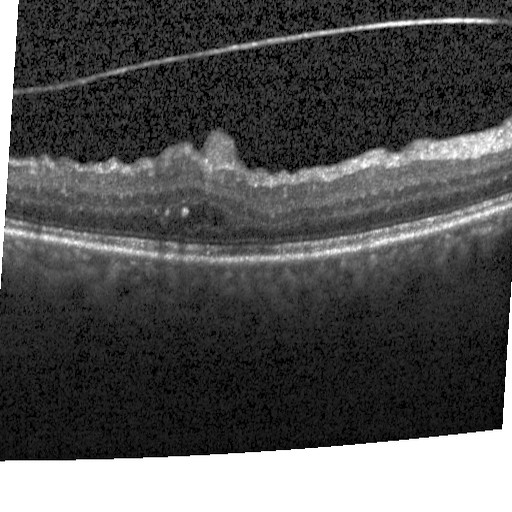
OCT line scan.
Assessment: diabetic macular edema (DME).